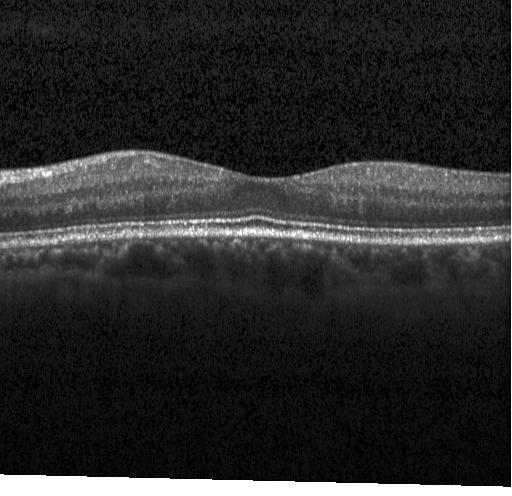
Macular OCT demonstrating no evidence of choroidal neovascularization, diabetic macular edema, or drusen.